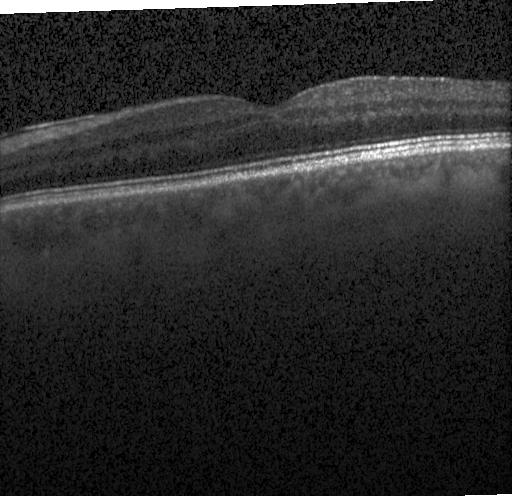

Macular scan · acquired on a Heidelberg Spectralis · OCT line scan. Diagnosis: no choroidal neovascularization, no diabetic macular edema, and no drusen.